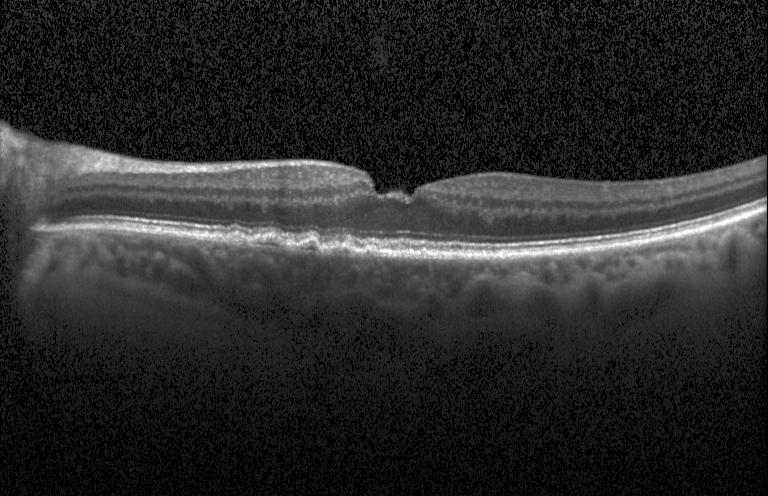

This B-scan demonstrates drusen.